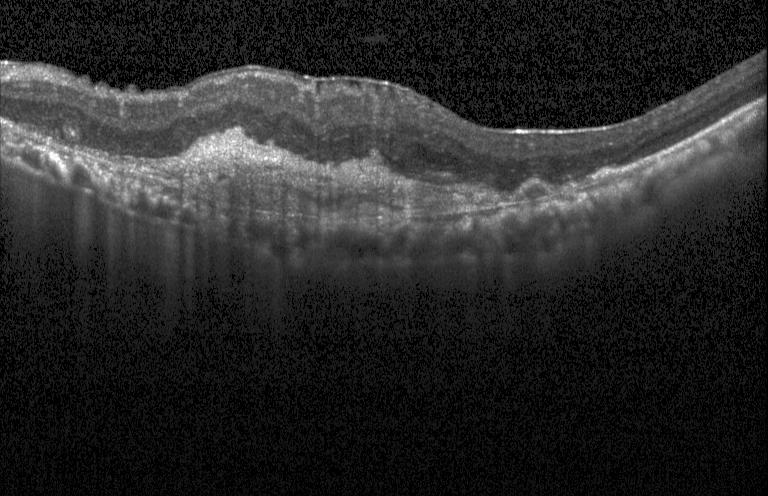 Finding: a choroidal neovascular membrane.